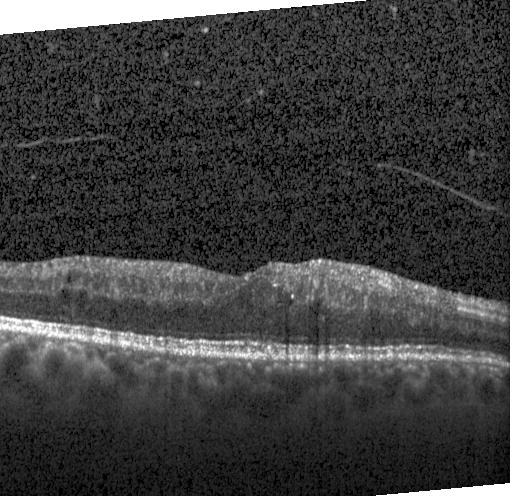
Retinal OCT cross-section. This B-scan demonstrates diabetic macular edema.